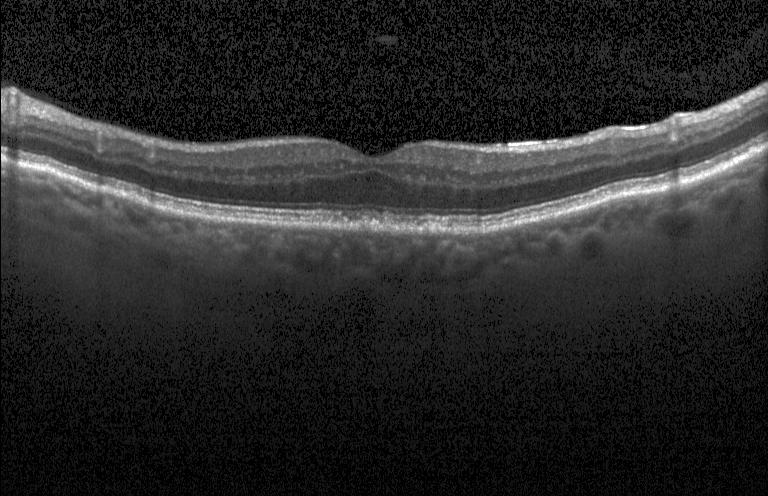 Retinal OCT cross-section — Assessment: no choroidal neovascularization, no diabetic macular edema, and no drusen.